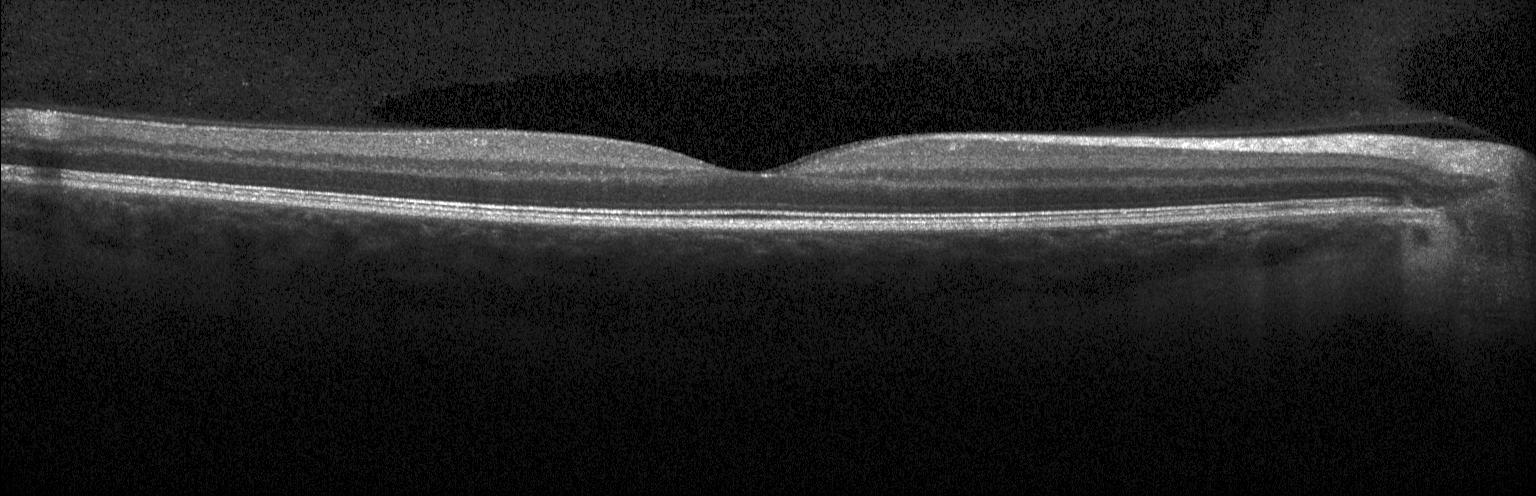
Spectral-domain OCT B-scan: no choroidal neovascularization, diabetic macular edema, or drusen.